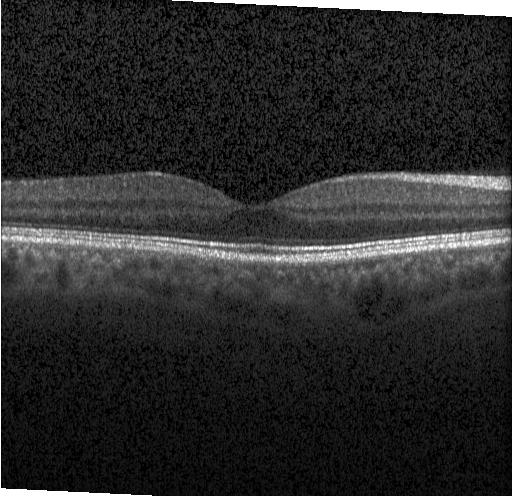
Spectral-domain OCT; retinal OCT cross-section
Finding: neither choroidal neovascularization, diabetic macular edema, nor drusen.